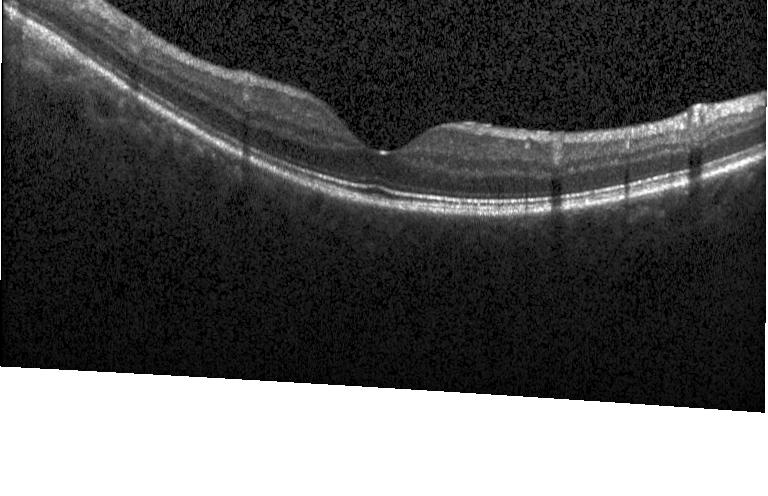

Fovea-centered. Spectral-domain optical coherence tomography. Optical coherence tomography scan. Instrument: Heidelberg Spectralis — OCT finding: no evidence of CNV, DME, or drusen.